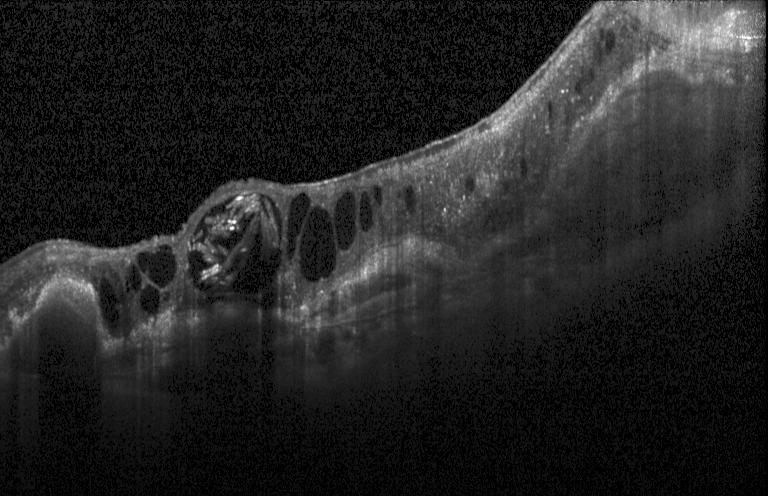

Diagnosis: choroidal neovascularization (CNV).